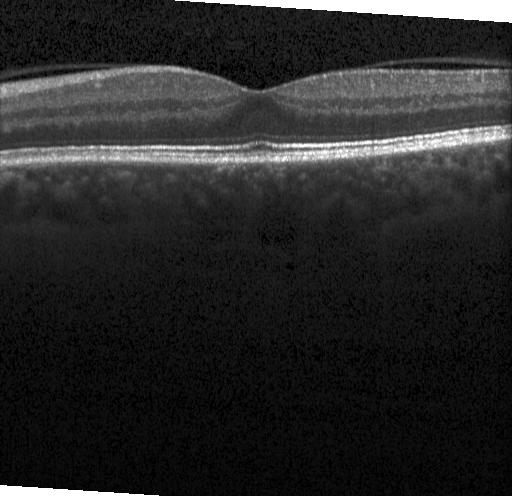

Optical coherence tomography scan — Finding: no evidence of CNV, DME, or drusen.